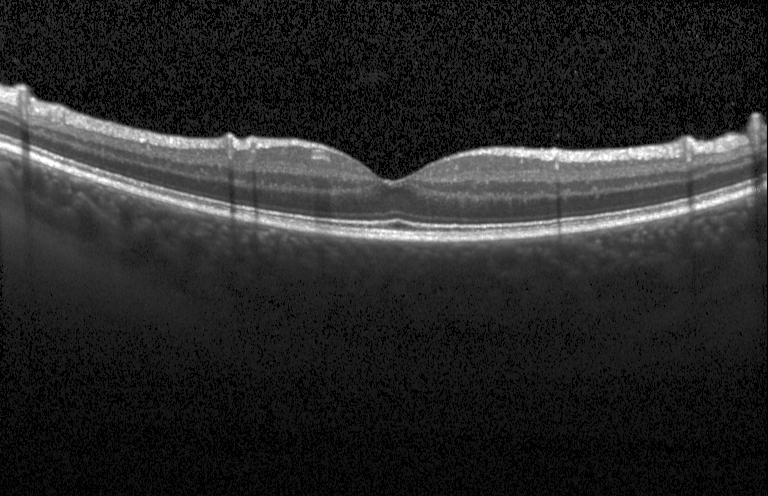
Instrument: Heidelberg Spectralis; optical coherence tomography scan; fovea-centered
Finding: no CNV, DME, or drusen.